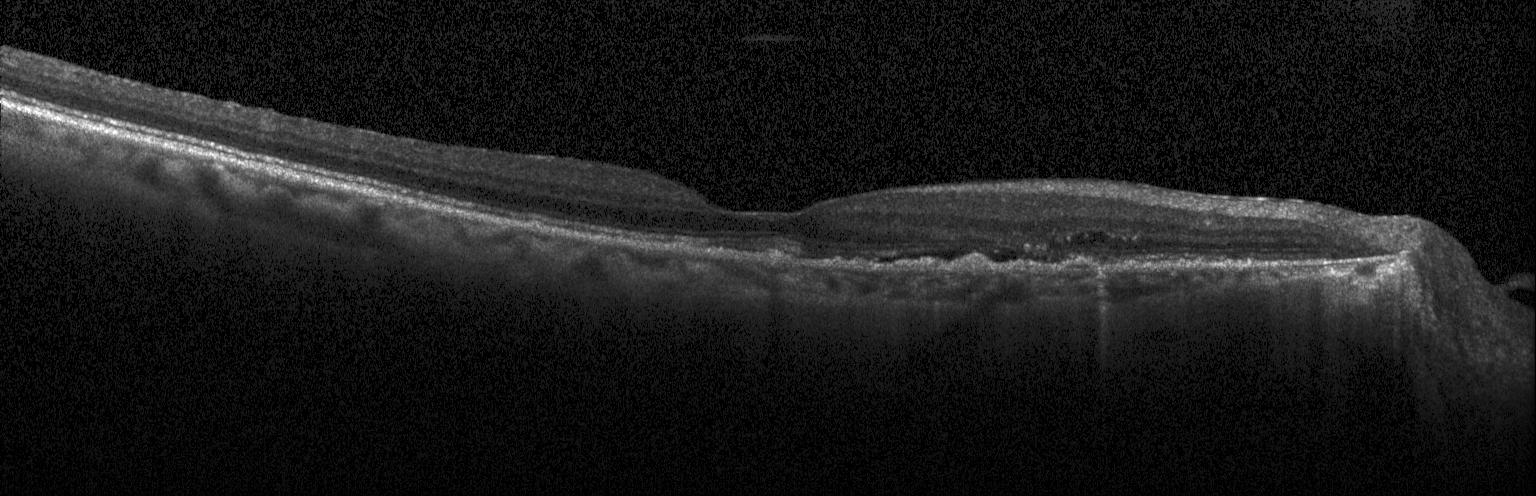

Diagnosis: choroidal neovascularization (CNV).